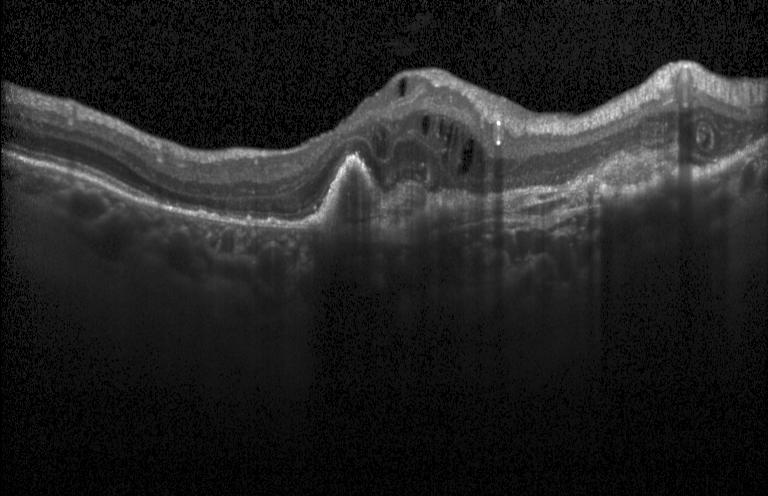

Finding: choroidal neovascularization.